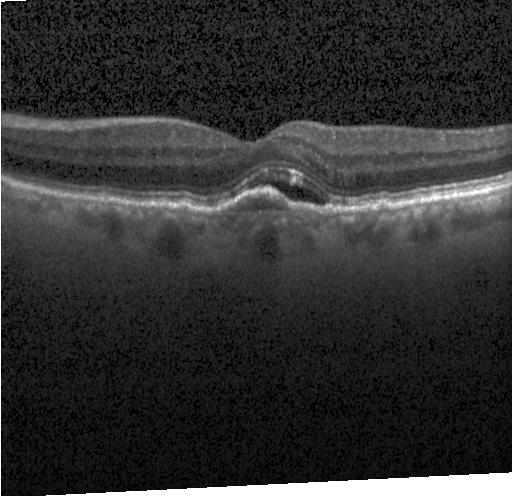

Spectral-domain OCT. Heidelberg Spectralis. Centered on the fovea. Retinal OCT cross-section.
OCT finding: a choroidal neovascular membrane.